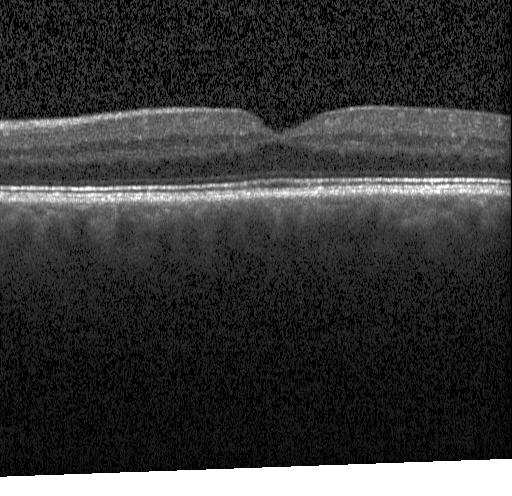

Retinal OCT cross-section
This B-scan demonstrates no evidence of choroidal neovascularization, diabetic macular edema, or drusen.